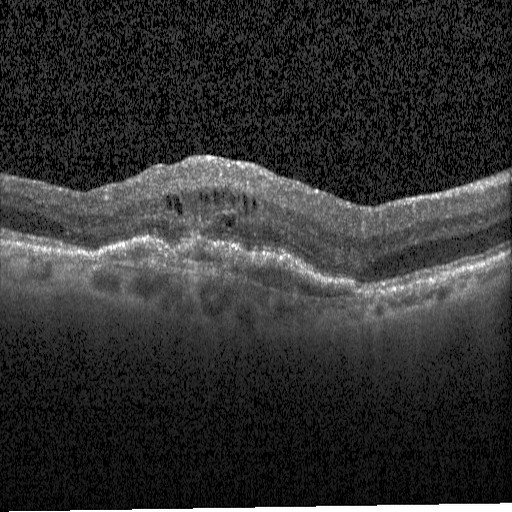 Horizontal scan through the fovea, instrument: Heidelberg Spectralis, optical coherence tomography scan, spectral-domain optical coherence tomography — This B-scan demonstrates DME.